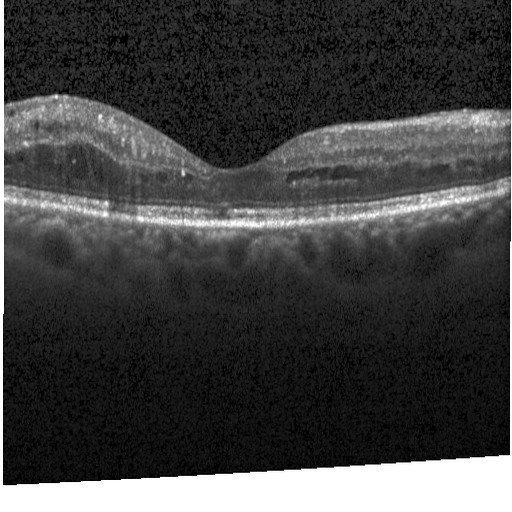 Impression: diabetic macular edema.